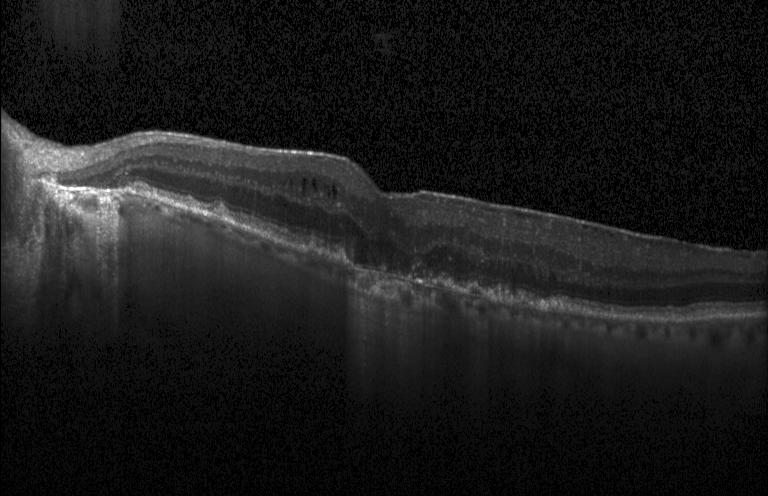

OCT B-scan · Heidelberg Spectralis.
The scan shows CNV.